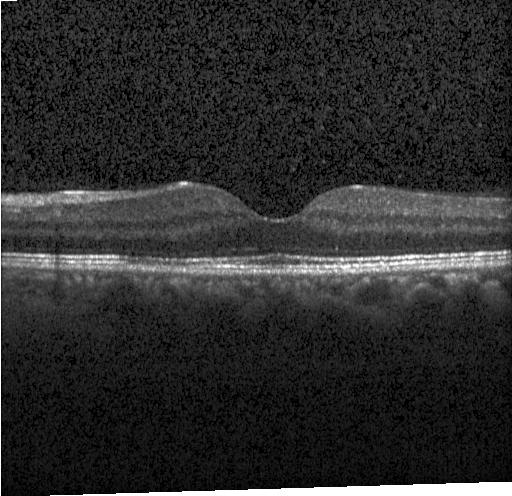 Spectral-domain optical coherence tomography · acquired on a Heidelberg Spectralis · optical coherence tomography scan — Finding: neither choroidal neovascularization, diabetic macular edema, nor drusen.